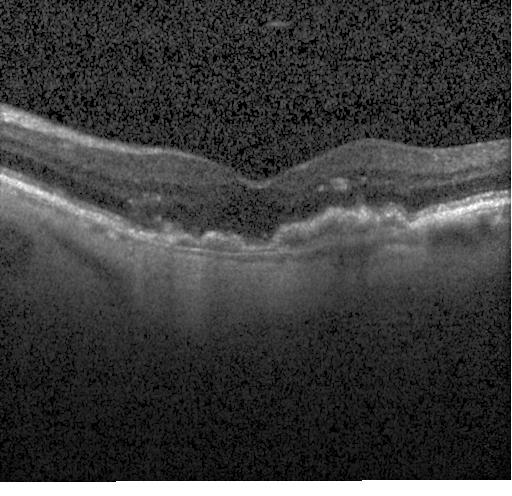
Centered on the fovea. Optical coherence tomography scan.
Diagnosis: a choroidal neovascular membrane.